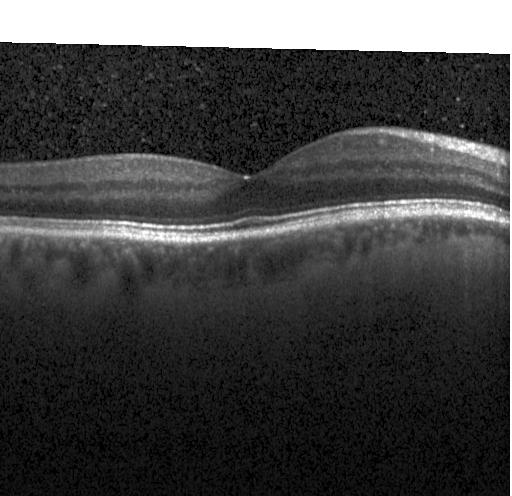
OCT line scan; through the macula. Macular OCT: neither choroidal neovascularization, diabetic macular edema, nor drusen.